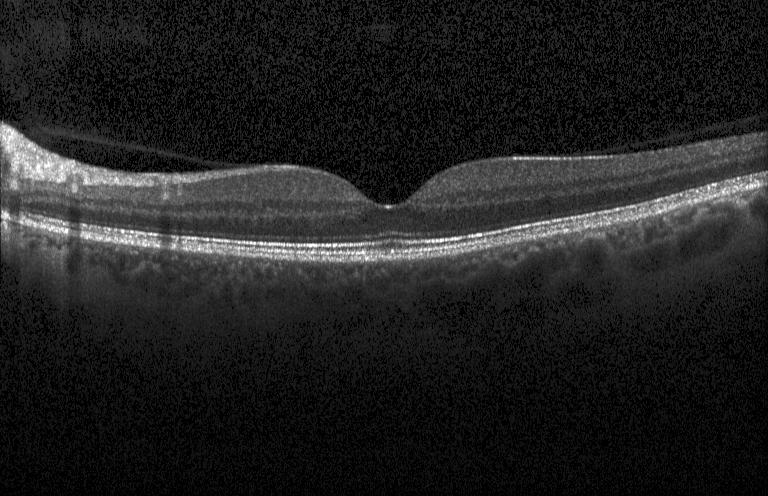 Spectral-domain OCT B-scan: no CNV, DME, or drusen.